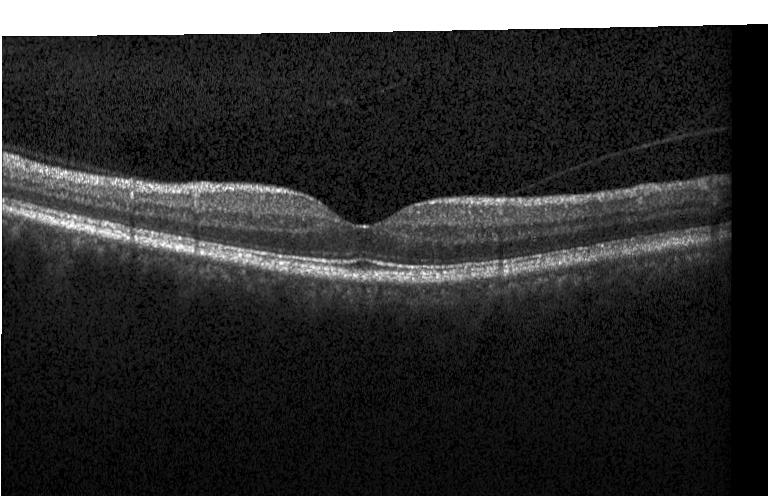

Dx: no evidence of CNV, DME, or drusen.